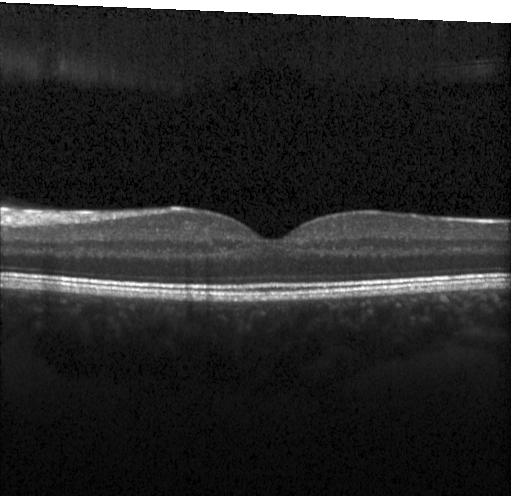
Dx: no CNV, DME, or drusen.